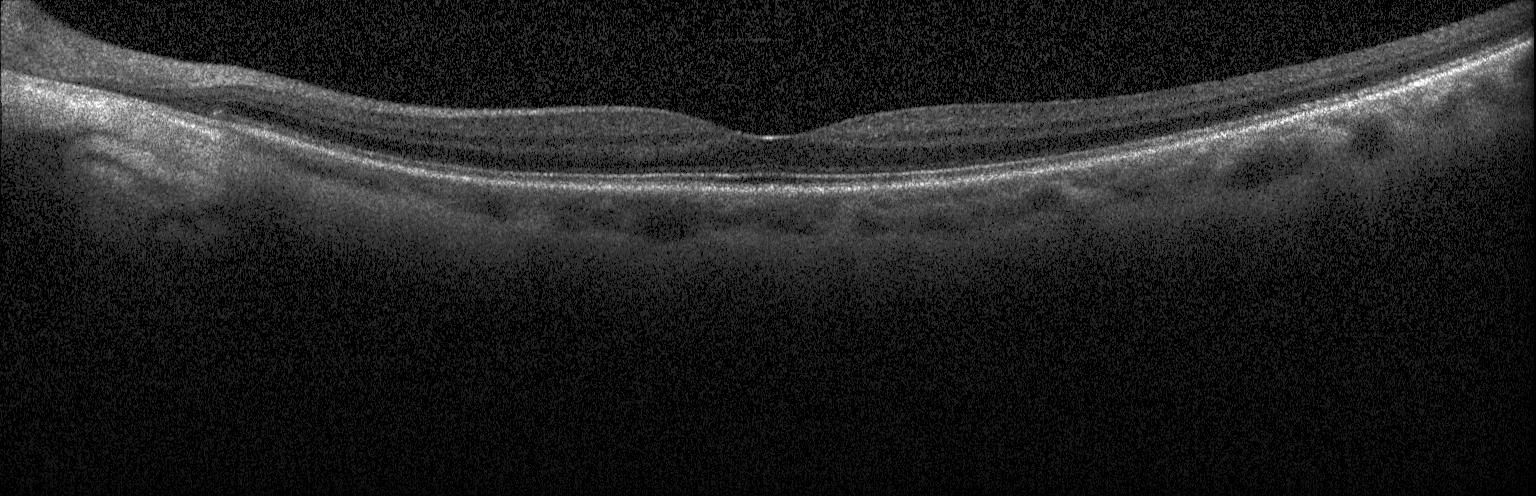 Horizontal scan through the fovea, OCT line scan.
Impression: no choroidal neovascularization, no diabetic macular edema, and no drusen.